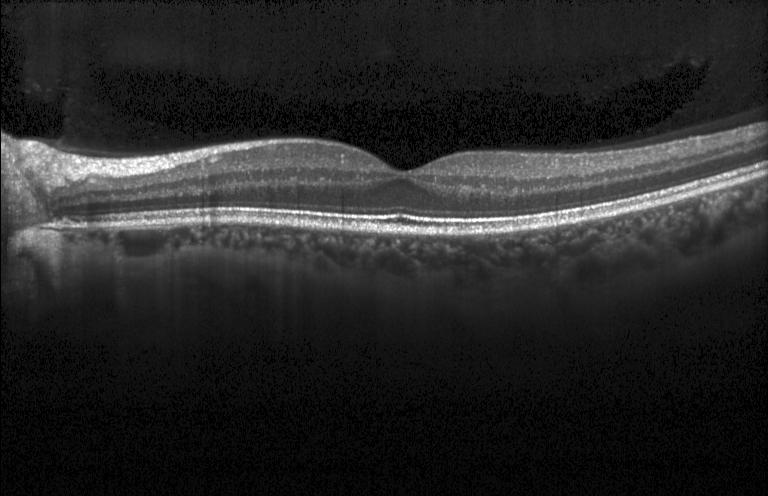
Spectral-domain OCT; OCT B-scan; fovea-centered
This B-scan demonstrates no CNV, no DME, and no drusen.